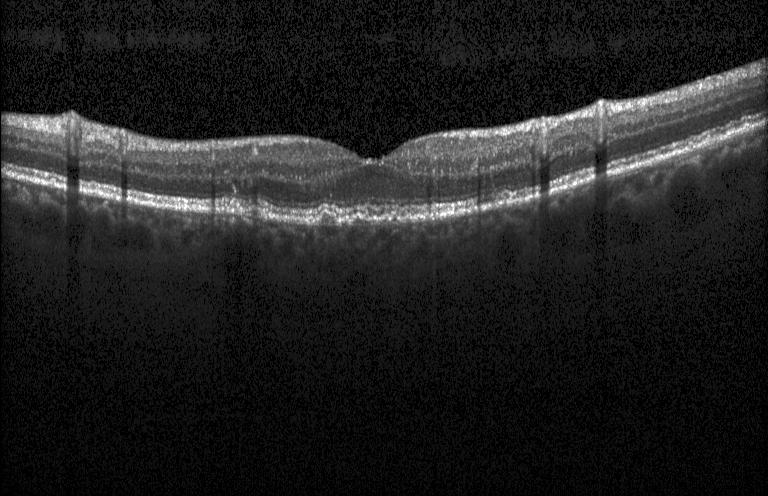
Diagnosis: drusen.